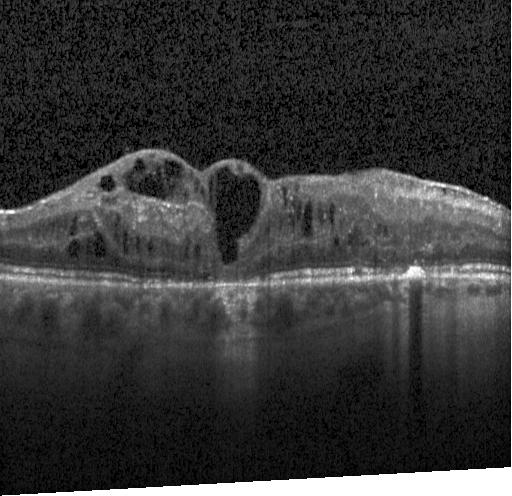
Retinal OCT B-scan. Acquired on a Heidelberg Spectralis. Impression: diabetic macular edema (DME).